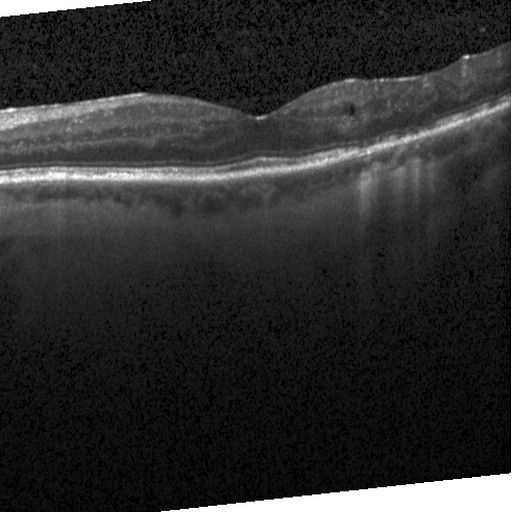

OCT finding: diabetic macular edema (DME).